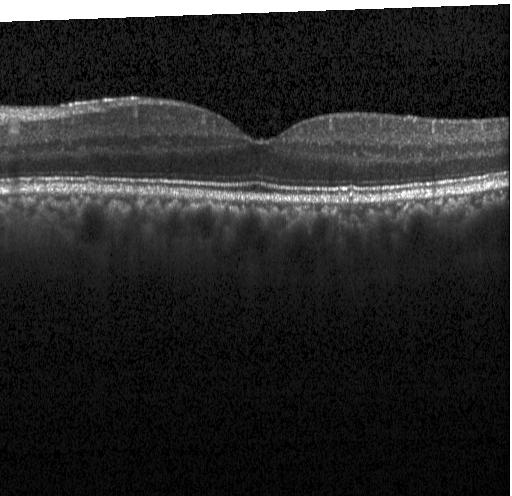 Assessment: drusen.